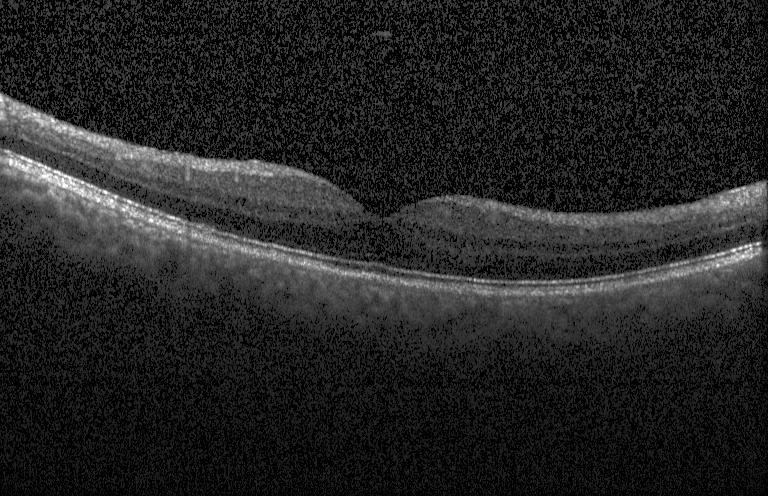
Impression: neither choroidal neovascularization, diabetic macular edema, nor drusen.